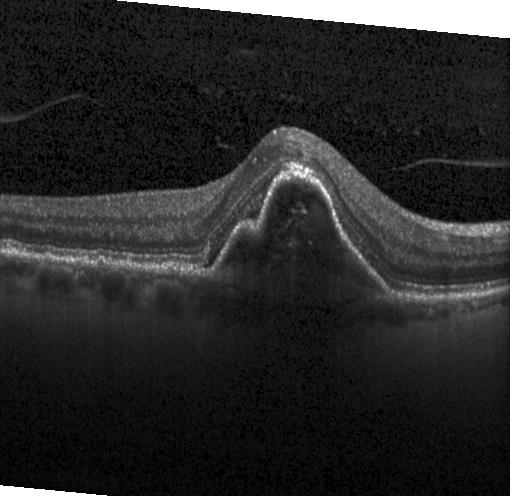
Retinal OCT B-scan; macular scan. Assessment: CNV.